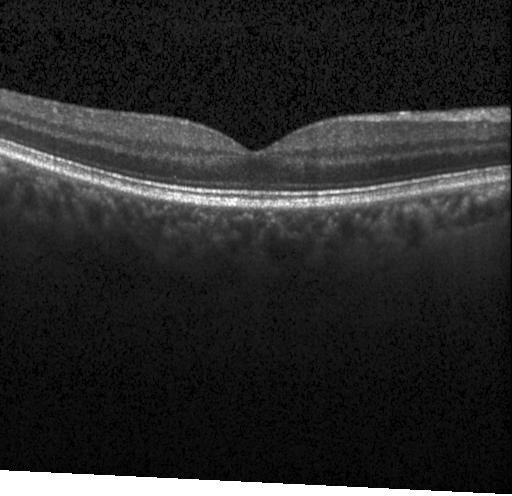
Optical coherence tomography scan.
Assessment: no evidence of choroidal neovascularization, diabetic macular edema, or drusen.